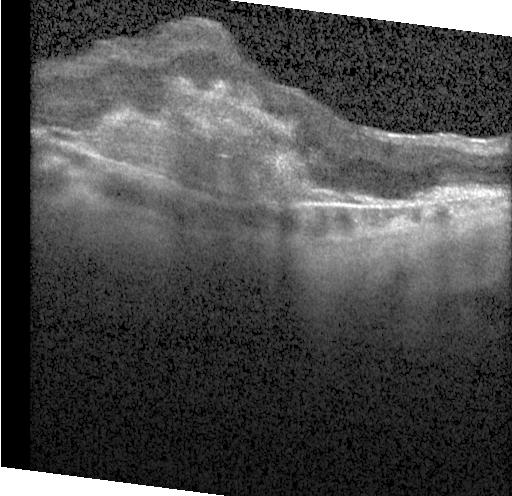

Impression: choroidal neovascularization.